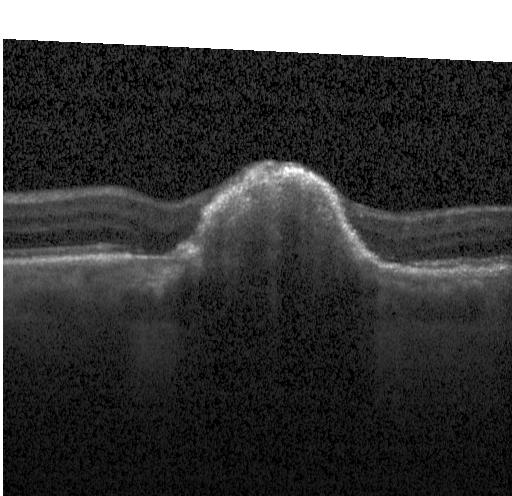
Macular OCT: choroidal neovascularization (CNV).